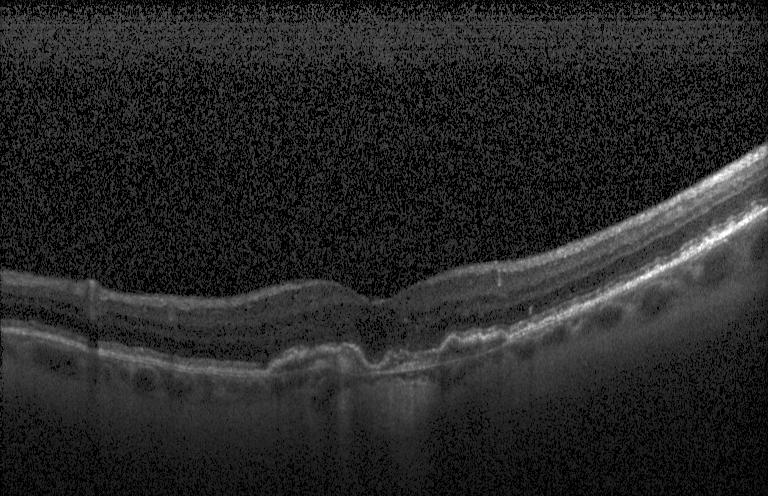 OCT line scan · acquired on a Heidelberg Spectralis.
Impression: a choroidal neovascular membrane.